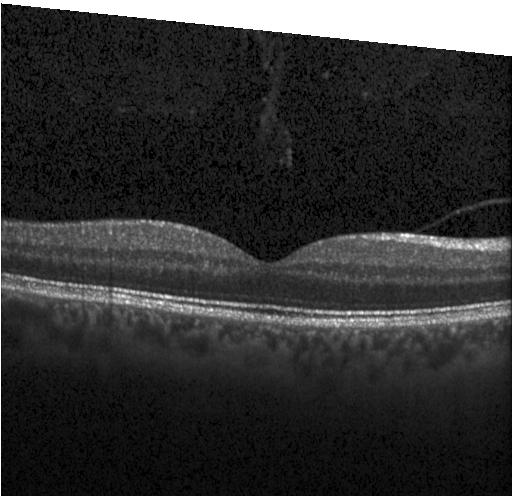

OCT B-scan, fovea-centered, spectral-domain OCT.
Assessment: no CNV, DME, or drusen.